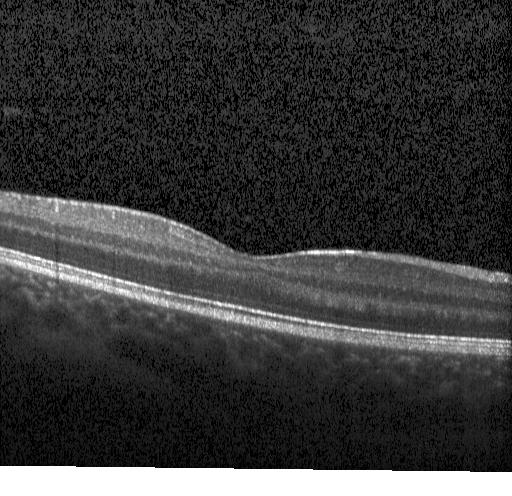
Retinal OCT B-scan. OCT finding: no evidence of choroidal neovascularization, diabetic macular edema, or drusen.